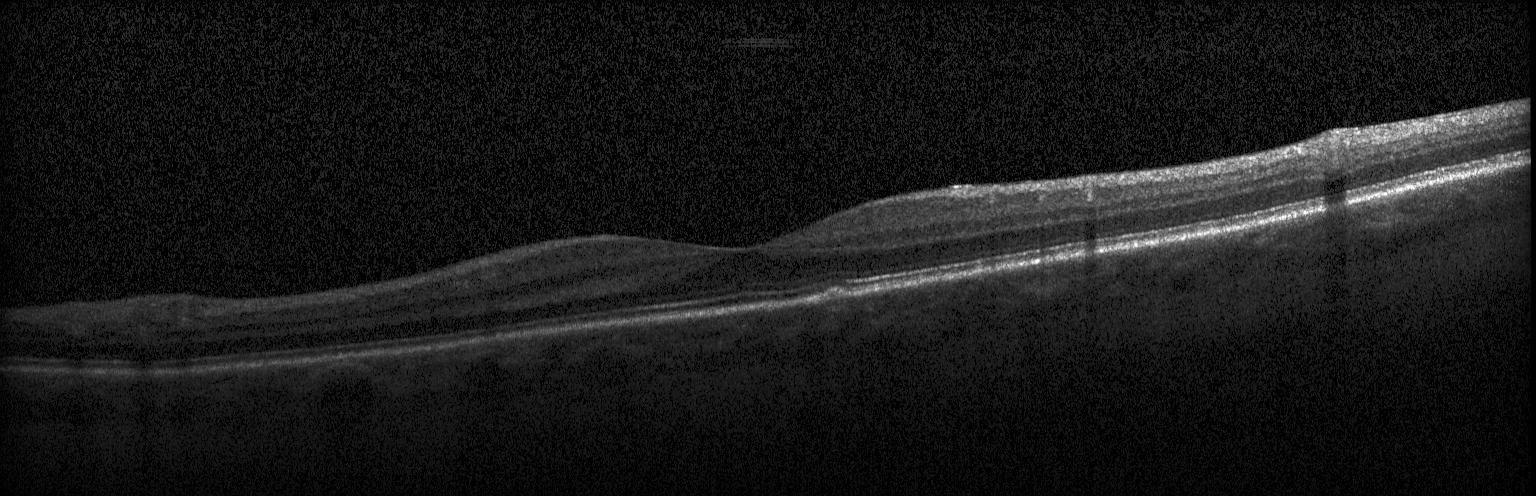

Optical coherence tomography scan · fovea-centered
The scan shows drusen.